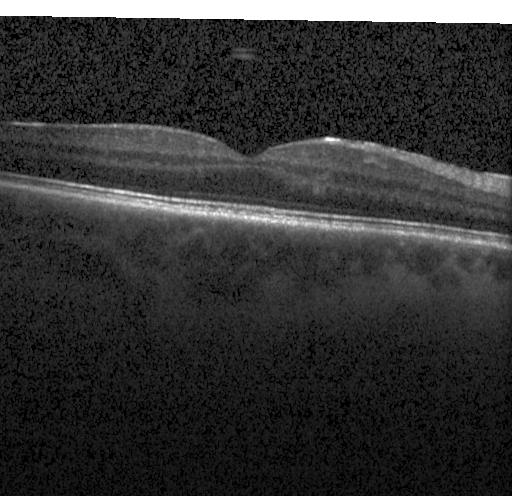

Spectral-domain OCT B-scan: no evidence of choroidal neovascularization, diabetic macular edema, or drusen.